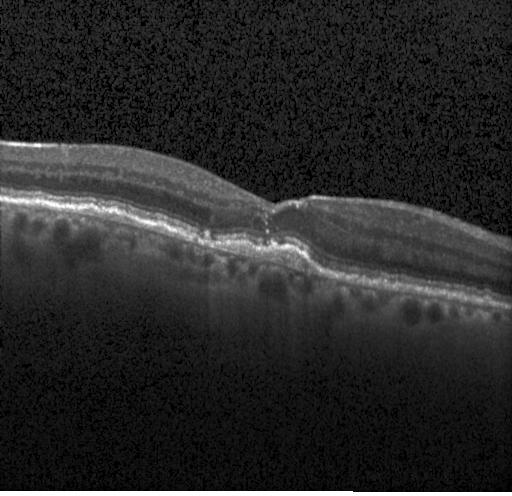 OCT scan showing CNV.